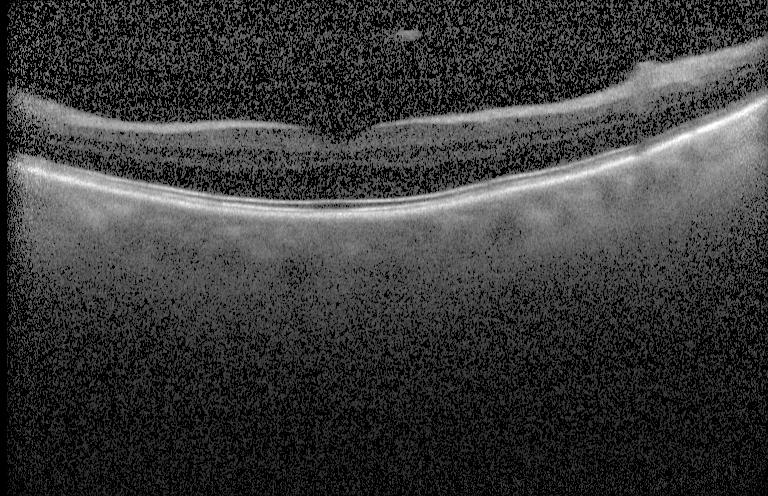
No choroidal neovascularization, diabetic macular edema, or drusen.